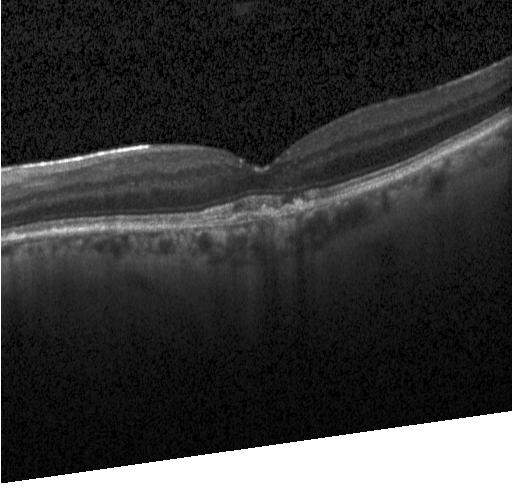

Spectral-domain optical coherence tomography. Centered on the fovea. Retinal OCT B-scan. Heidelberg Spectralis OCT system — Assessment: a choroidal neovascular membrane.